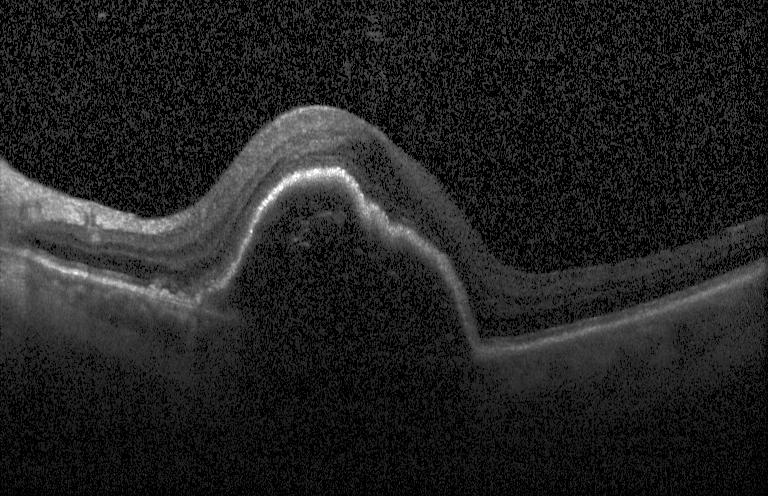
Spectral-domain optical coherence tomography. Optical coherence tomography B-scan — Assessment: CNV.